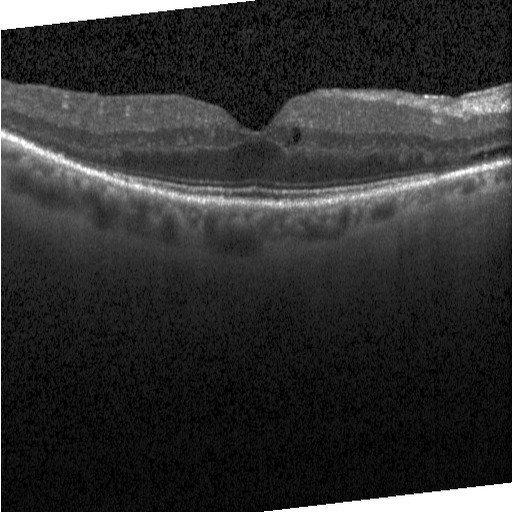

Spectral-domain OCT B-scan: diabetic macular edema (DME).